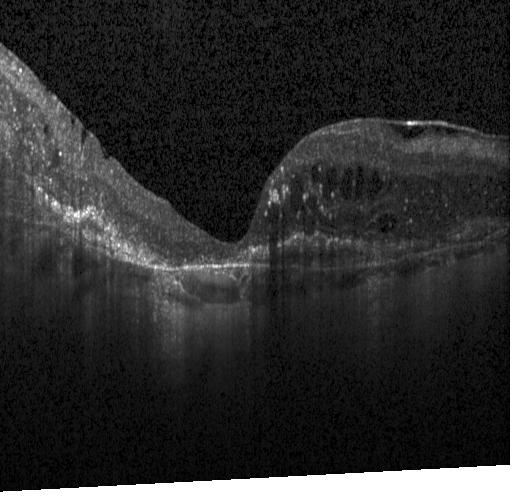

Assessment: choroidal neovascularization (CNV).